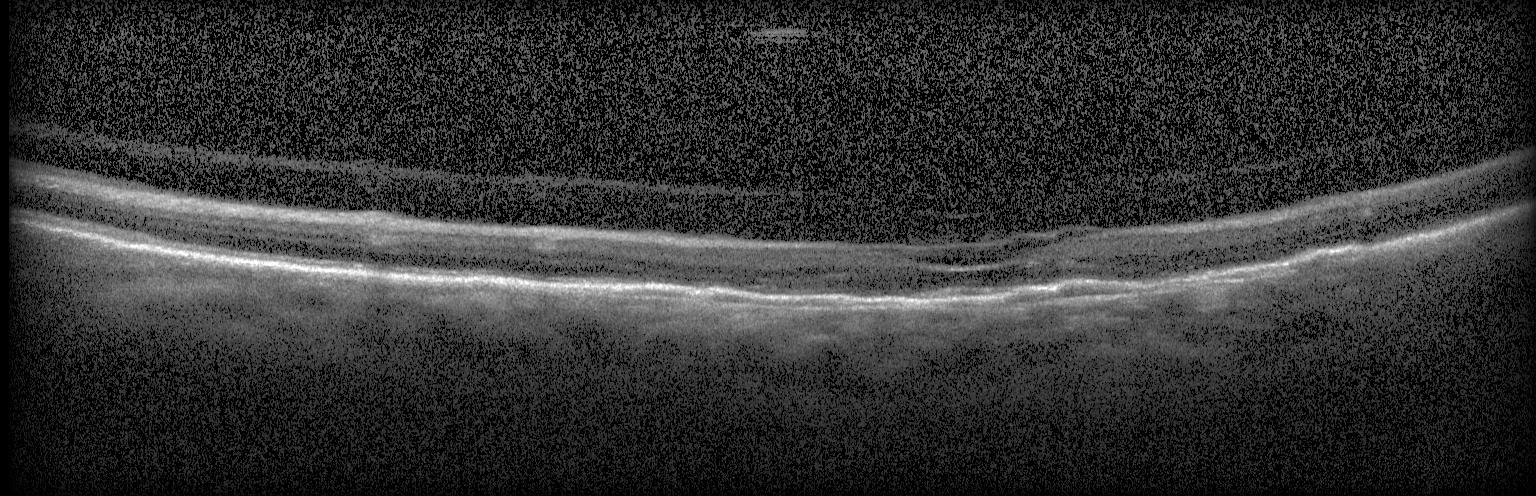

Optical coherence tomography scan; through the macula; acquired on a Heidelberg Spectralis; spectral-domain optical coherence tomography. Impression: a choroidal neovascular membrane.